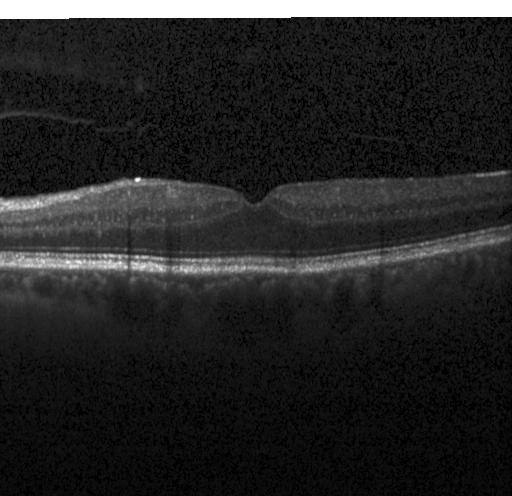 Fovea-centered, optical coherence tomography B-scan.
Assessment: no CNV, no DME, and no drusen.